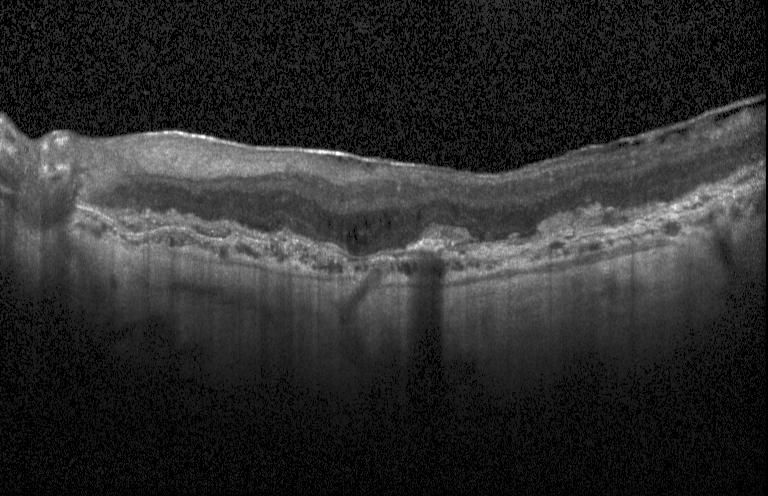
Spectral-domain OCT B-scan: choroidal neovascularization.